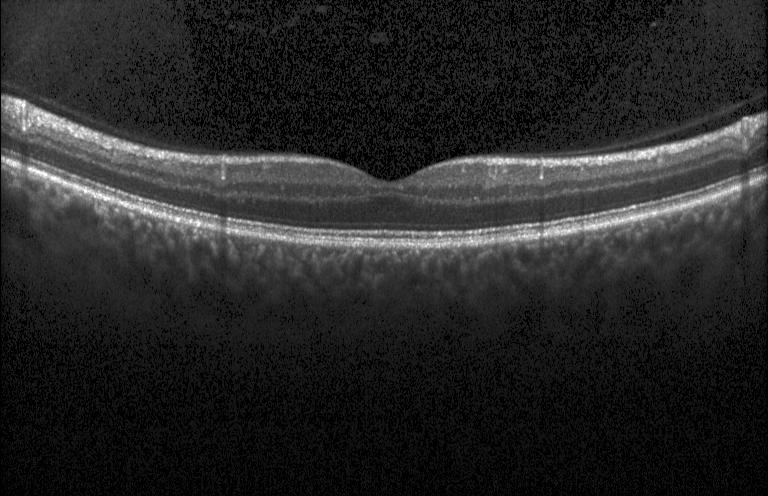
The scan shows no evidence of choroidal neovascularization, diabetic macular edema, or drusen.